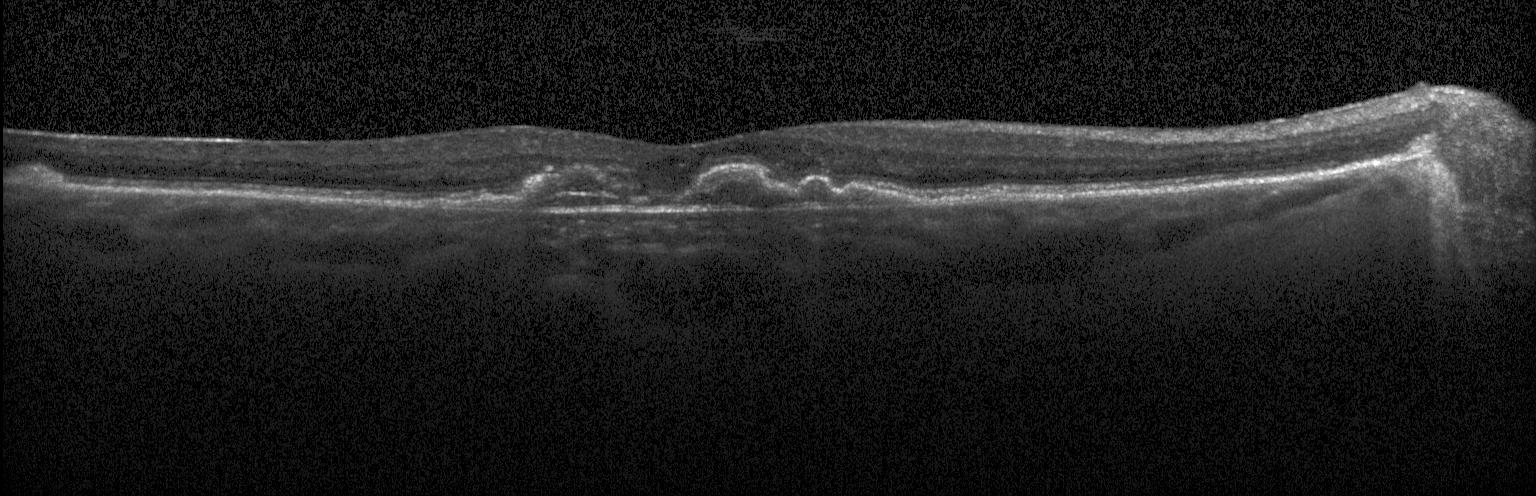 Retinal OCT B-scan
OCT finding: a choroidal neovascular membrane.